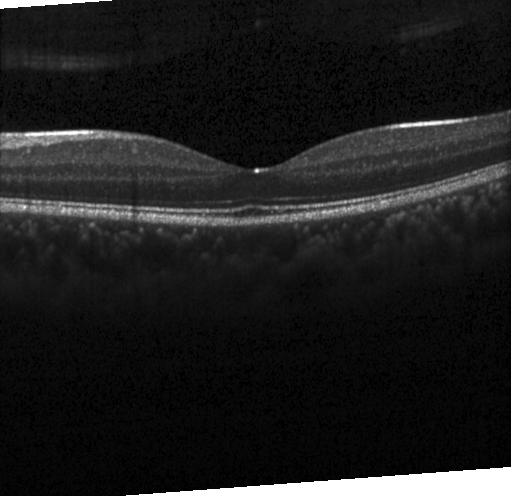

Optical coherence tomography B-scan; horizontal scan through the fovea
Finding: no choroidal neovascularization, no diabetic macular edema, and no drusen.